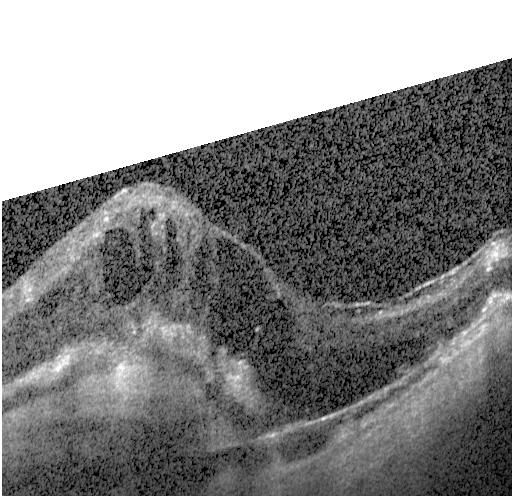

Optical coherence tomography B-scan; spectral-domain OCT; through the macula
Impression: CNV.